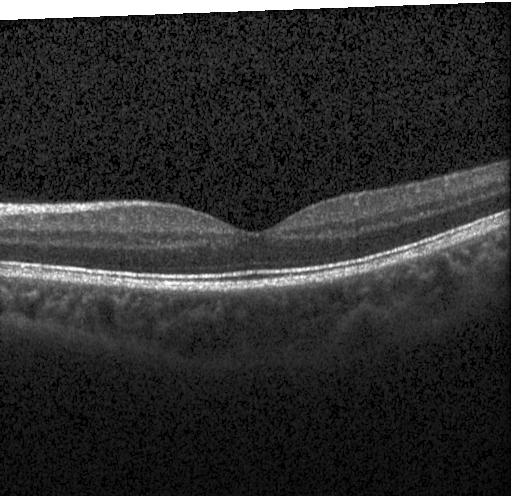

Macular OCT: neither CNV, DME, nor drusen.